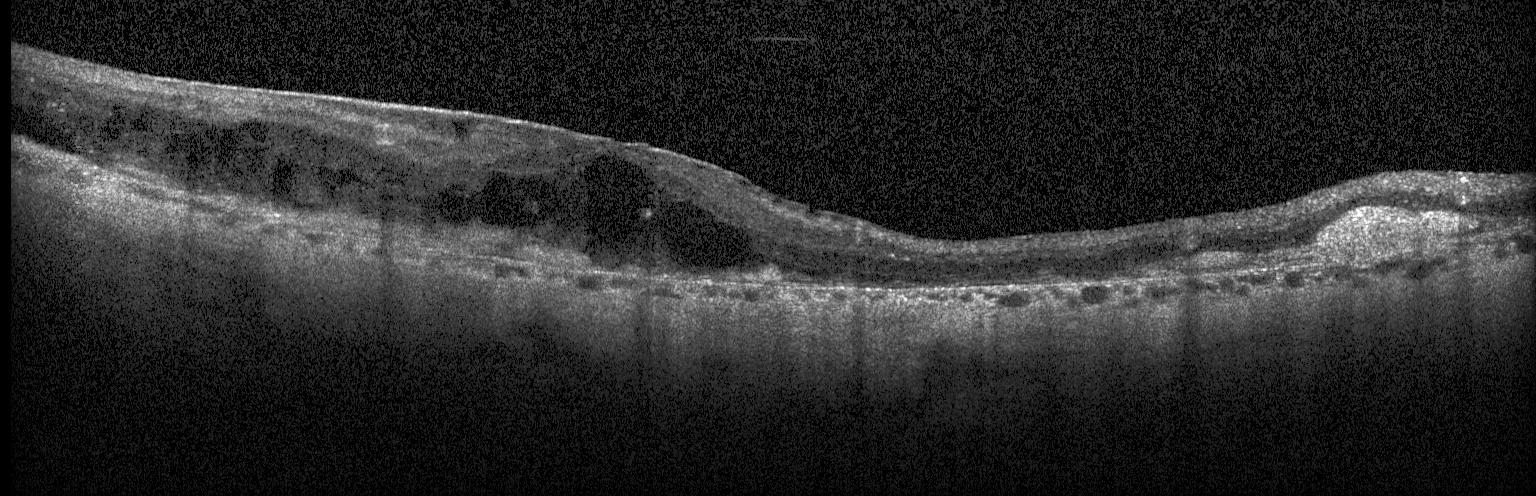
This B-scan demonstrates CNV.